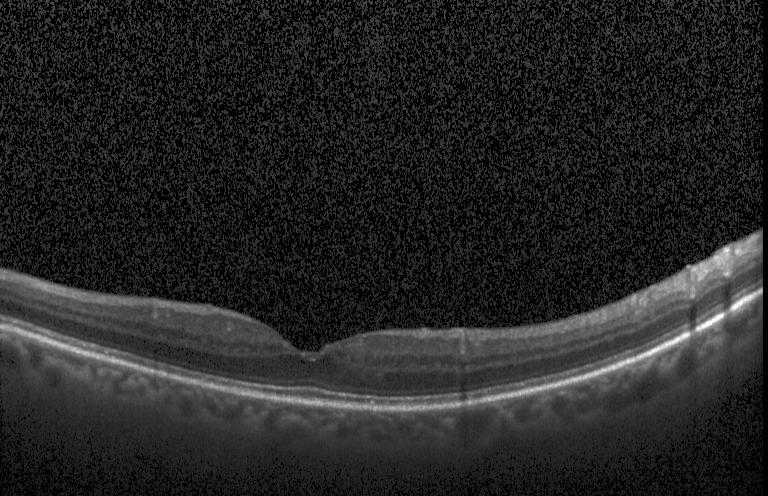 Retinal OCT B-scan, horizontal scan through the fovea
This B-scan demonstrates no CNV, no DME, and no drusen.